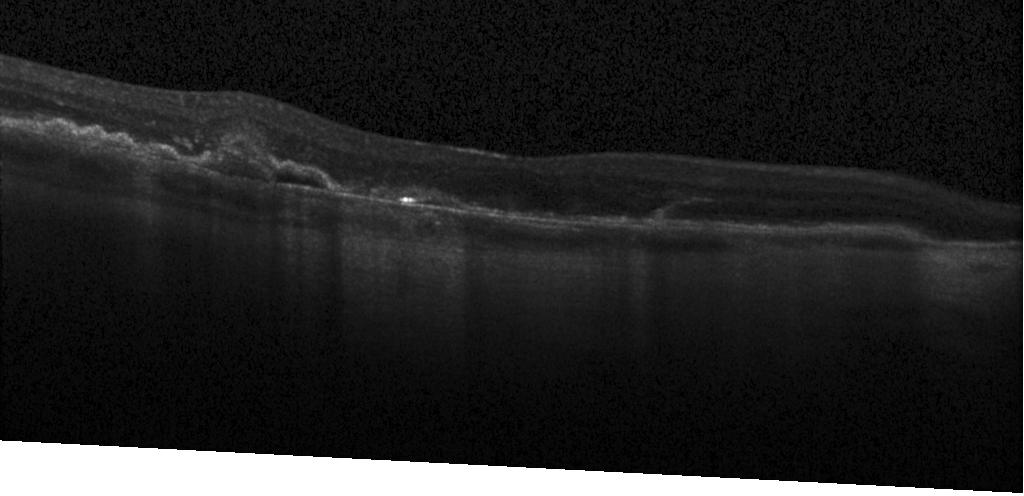
SD-OCT · through the macula · acquired on a Heidelberg Spectralis · retinal OCT B-scan. Macular OCT: CNV.